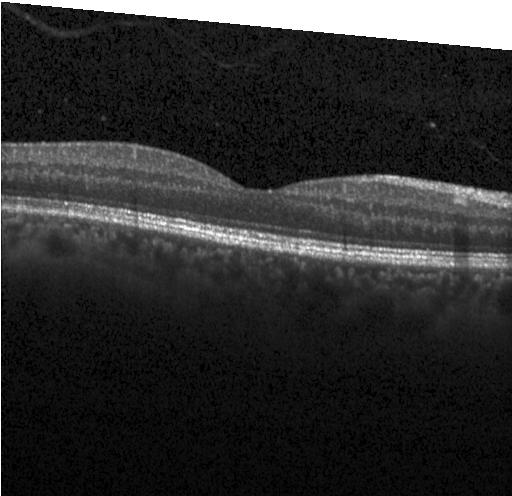

OCT B-scan
The scan shows neither CNV, DME, nor drusen.